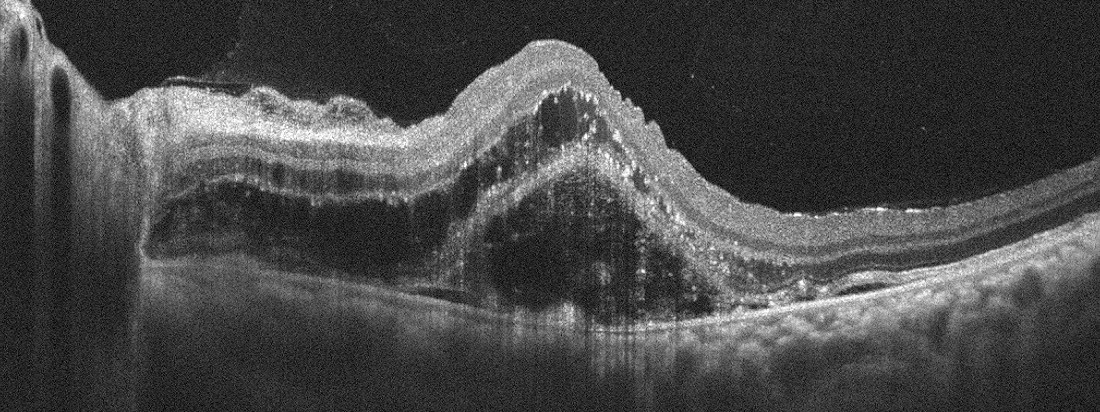

Optical coherence tomography B-scan · instrument: Optovue Avanti RTVue XR.
Assessment: retinal vein occlusion (RVO).